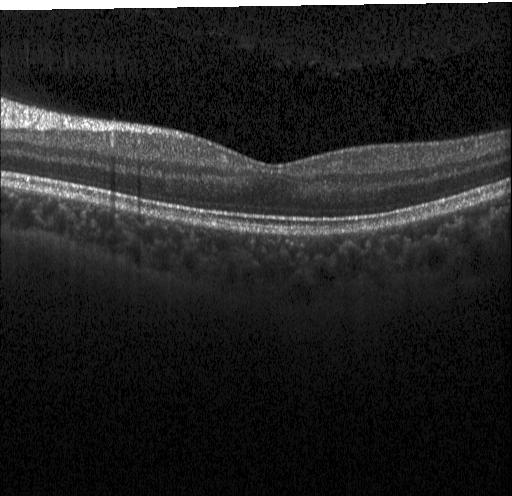
Macular OCT: no choroidal neovascularization, no diabetic macular edema, and no drusen.